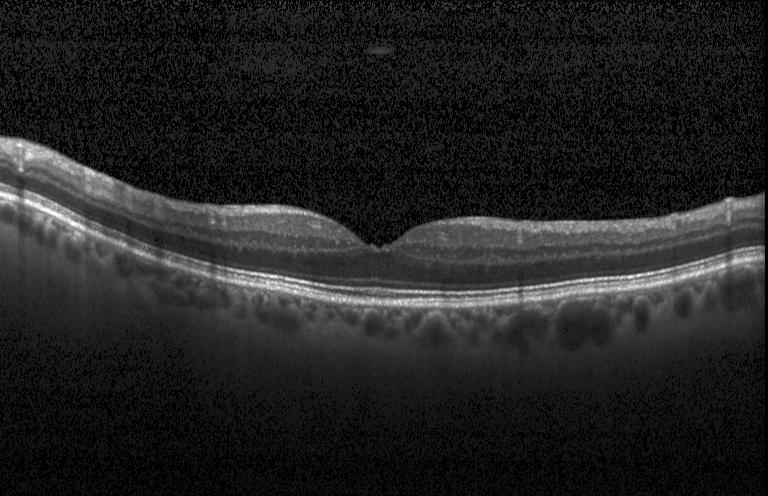
Instrument: Heidelberg Spectralis, retinal OCT cross-section, macular scan, spectral-domain optical coherence tomography.
No choroidal neovascularization, no diabetic macular edema, and no drusen.